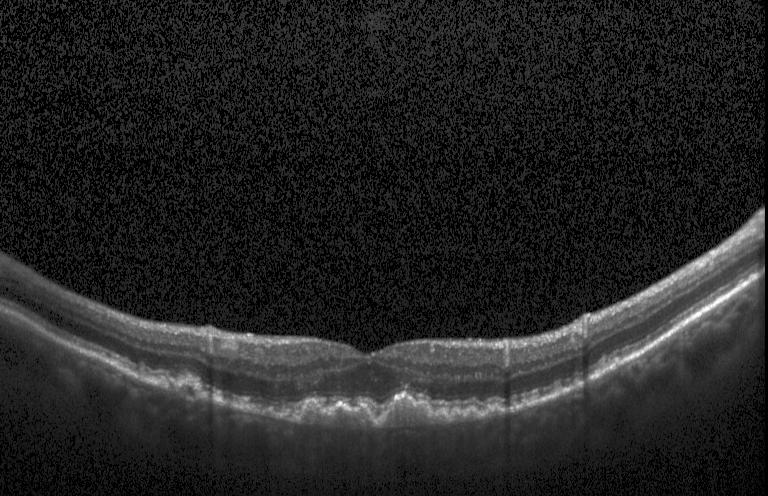 Retinal OCT cross-section.
This B-scan demonstrates sub-RPE drusenoid deposits.